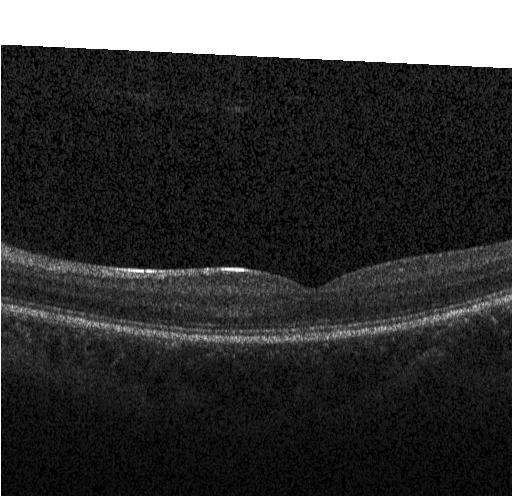
OCT B-scan · horizontal scan through the fovea · SD-OCT.
This B-scan demonstrates no choroidal neovascularization, diabetic macular edema, or drusen.